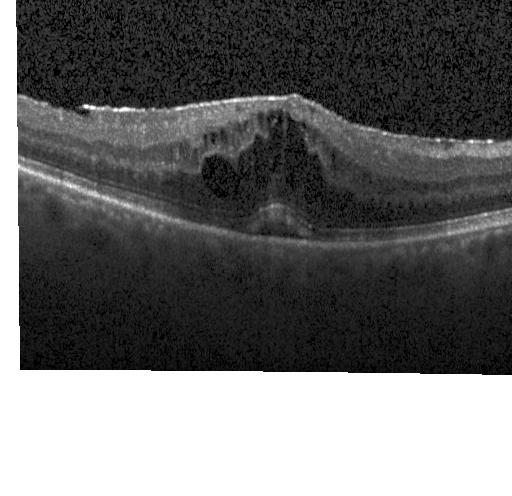

Retinal OCT B-scan · acquired on a Heidelberg Spectralis. DME.